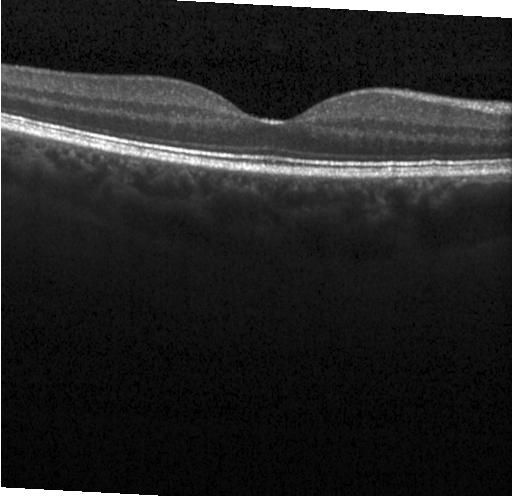

Horizontal scan through the fovea, OCT line scan, SD-OCT. This B-scan demonstrates no CNV, DME, or drusen.